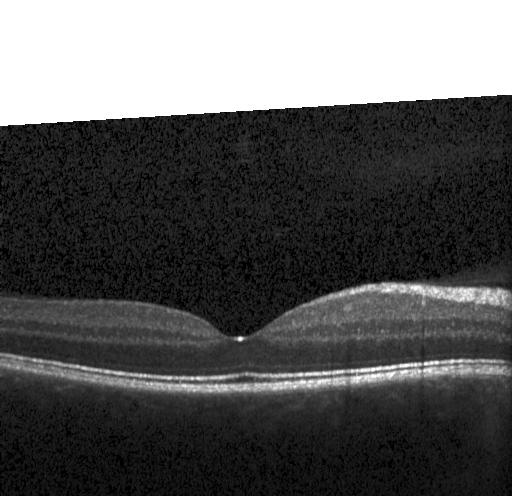
OCT B-scan
Diagnosis: no evidence of CNV, DME, or drusen.